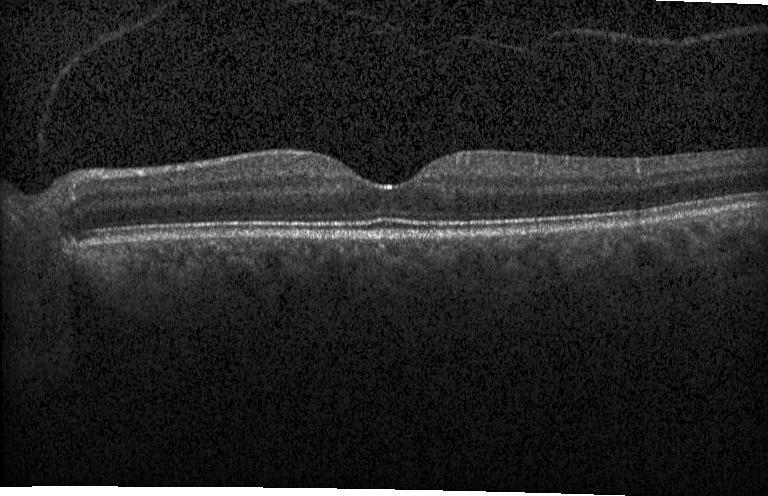 No choroidal neovascularization, diabetic macular edema, or drusen.